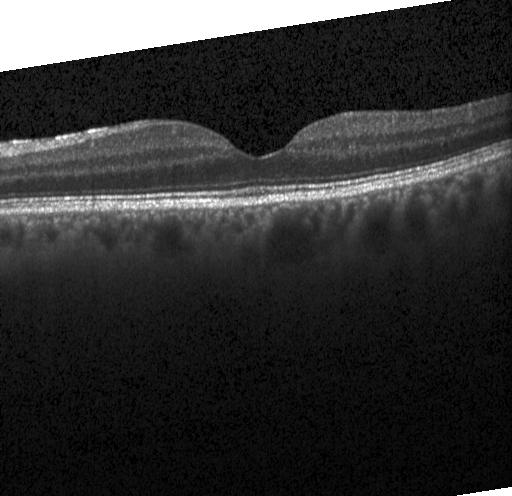 Finding: no choroidal neovascularization, no diabetic macular edema, and no drusen.